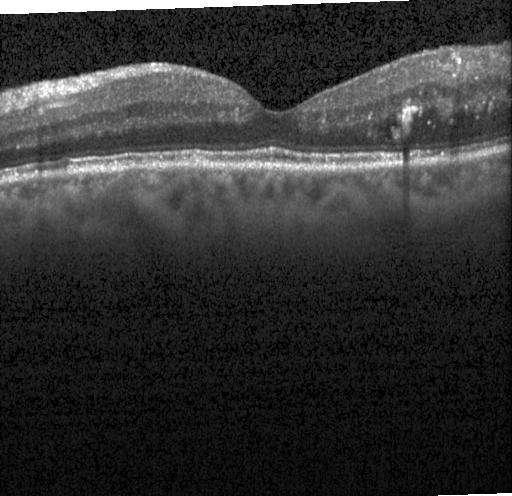

Finding: diabetic macular edema.